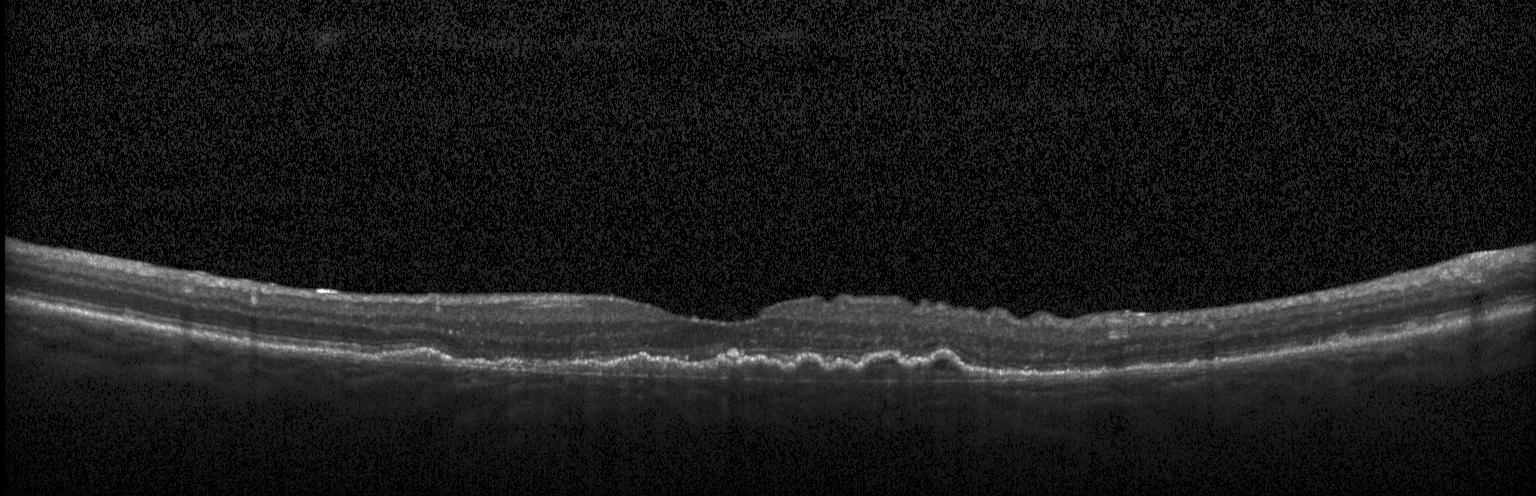

Assessment: choroidal neovascularization (CNV).